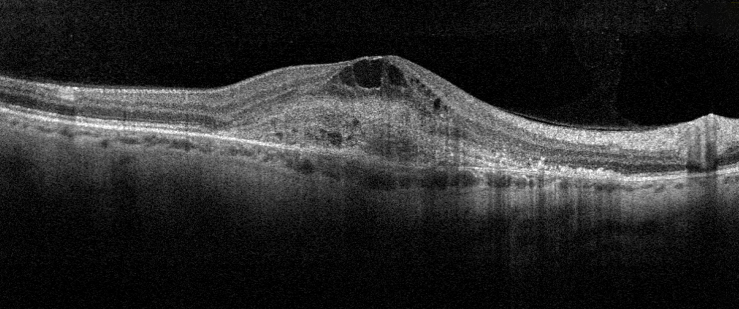 The scan shows AMD.